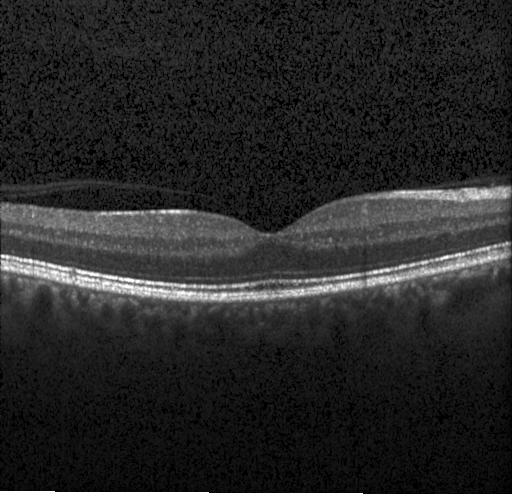

Macular OCT: no choroidal neovascularization, no diabetic macular edema, and no drusen.